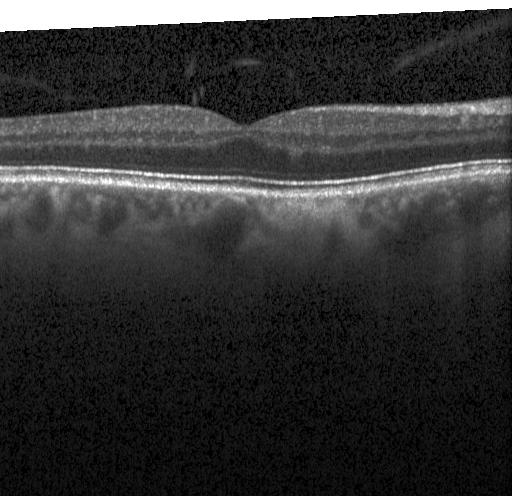 Retinal OCT cross-section, spectral-domain OCT, Heidelberg Spectralis OCT system, centered on the fovea. OCT finding: no evidence of choroidal neovascularization, diabetic macular edema, or drusen.